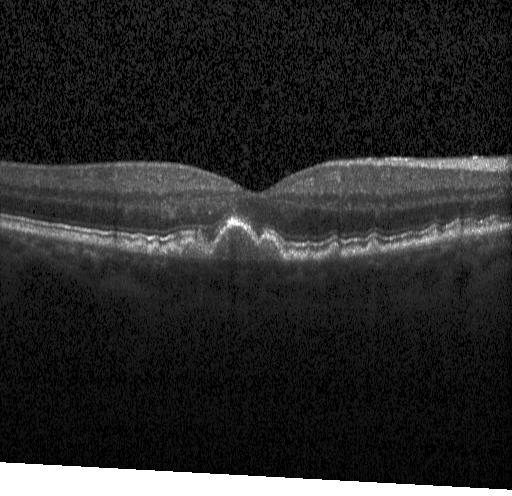
Impression: drusen.